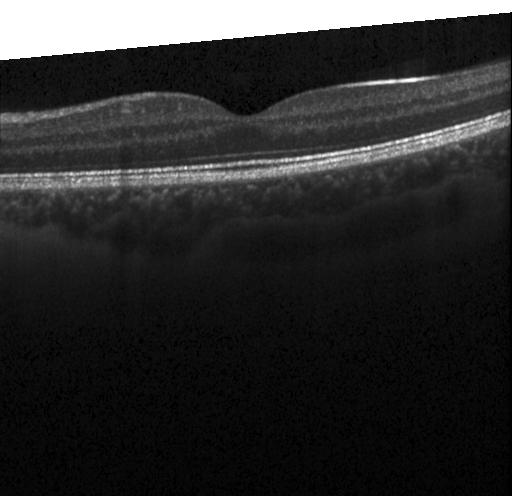 Instrument: Heidelberg Spectralis · OCT B-scan
Dx: no choroidal neovascularization, diabetic macular edema, or drusen.